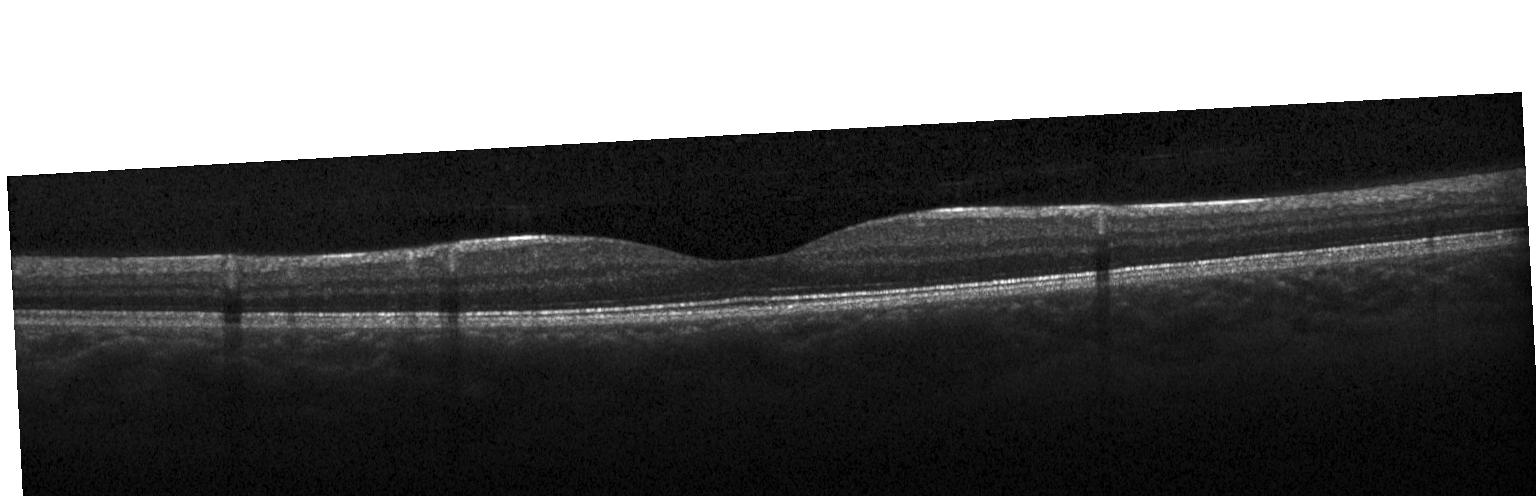

Spectral-domain OCT B-scan: neither choroidal neovascularization, diabetic macular edema, nor drusen.